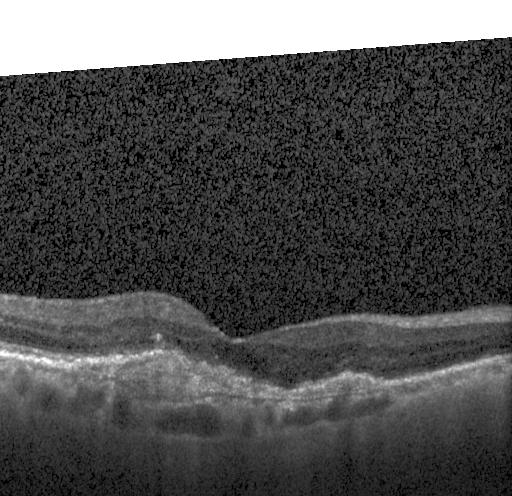

This B-scan demonstrates a choroidal neovascular membrane.